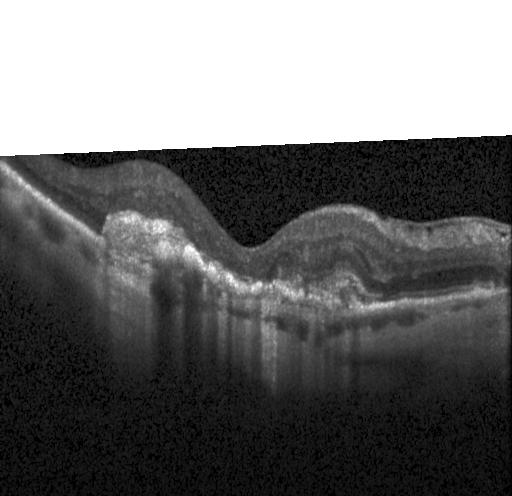
Spectral-domain OCT B-scan: choroidal neovascularization.